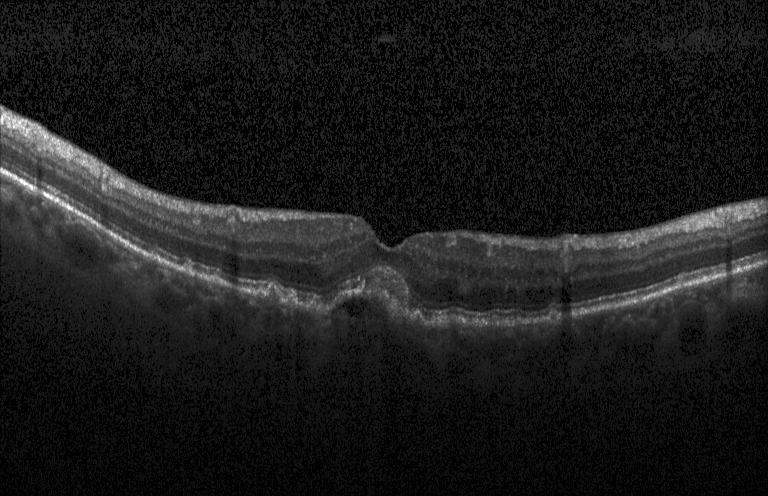
Diagnosis: a choroidal neovascular membrane.